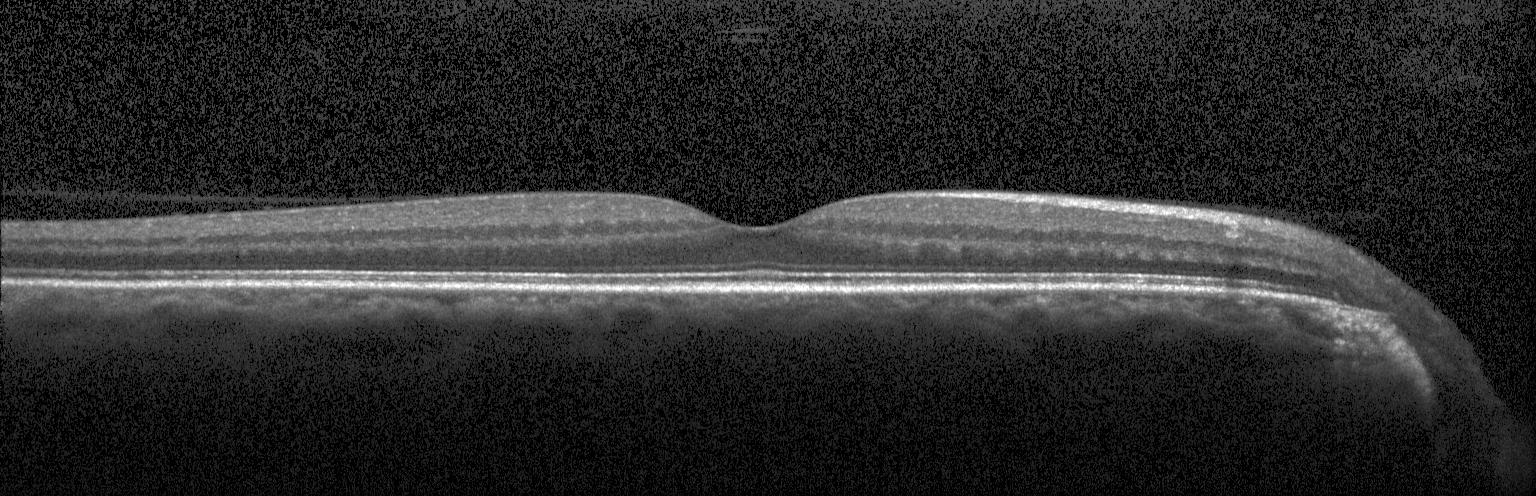
Finding: neither choroidal neovascularization, diabetic macular edema, nor drusen.